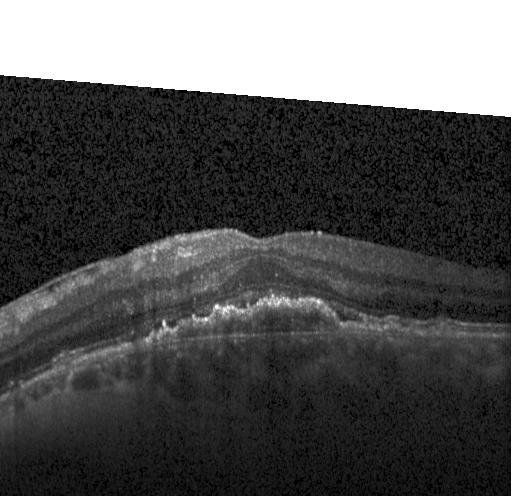
Retinal OCT cross-section; Heidelberg Spectralis OCT system; through the macula; spectral-domain OCT — The scan shows a choroidal neovascular membrane.